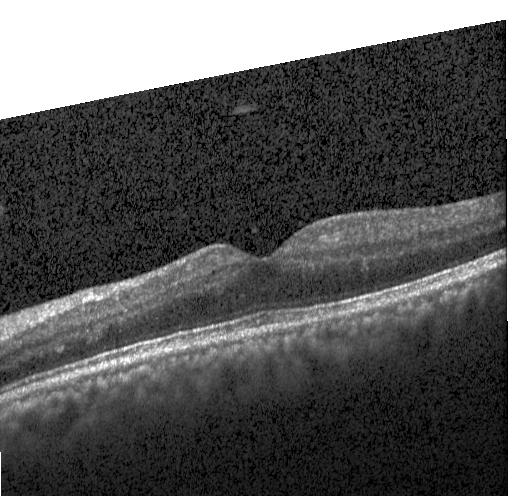
Retinal OCT cross-section, spectral-domain OCT — Assessment: no choroidal neovascularization, diabetic macular edema, or drusen.